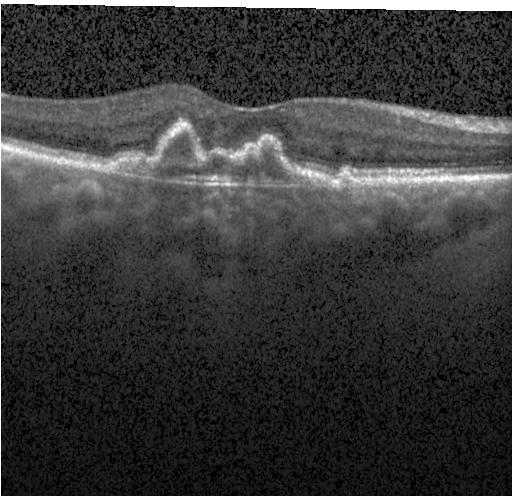
Macular OCT: a choroidal neovascular membrane.